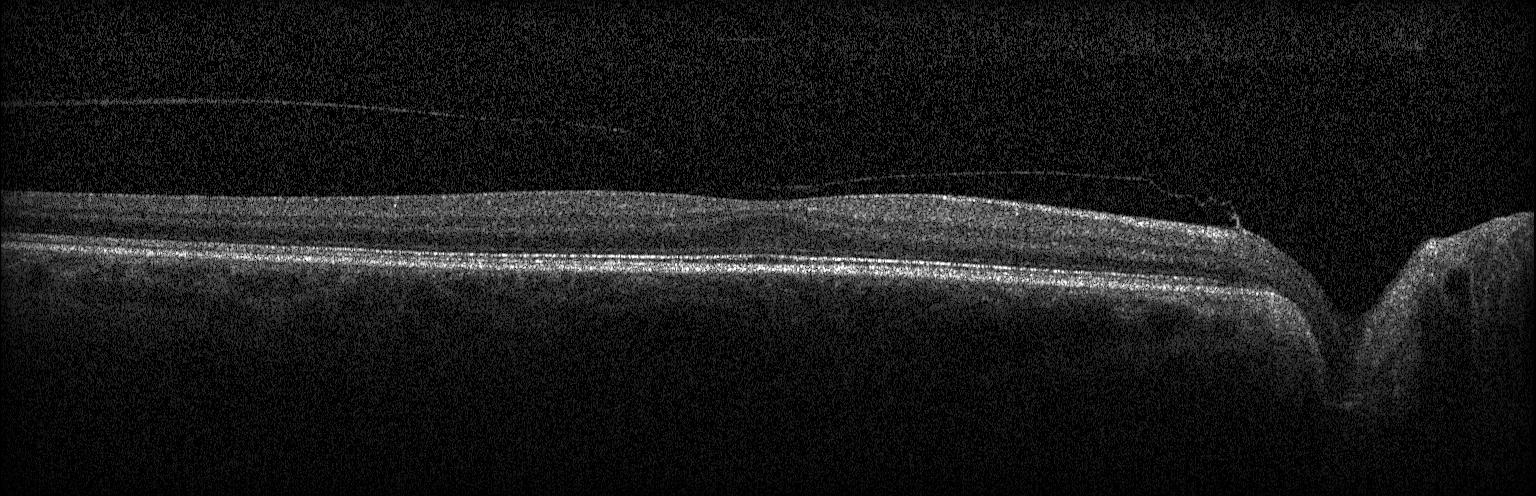

Impression: no choroidal neovascularization, diabetic macular edema, or drusen.